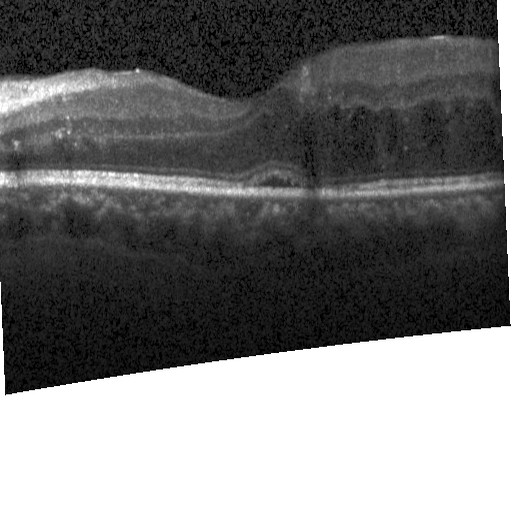 Centered on the fovea. Retinal OCT B-scan
The scan shows diabetic macular edema (DME).